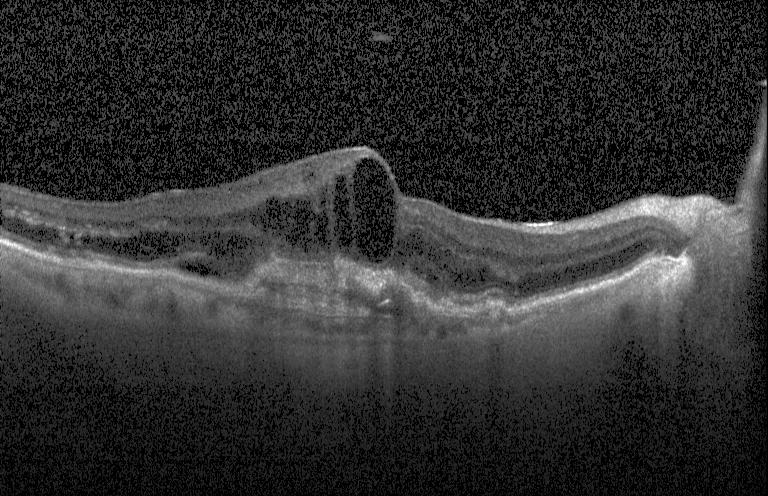
Macular OCT: choroidal neovascularization (CNV).